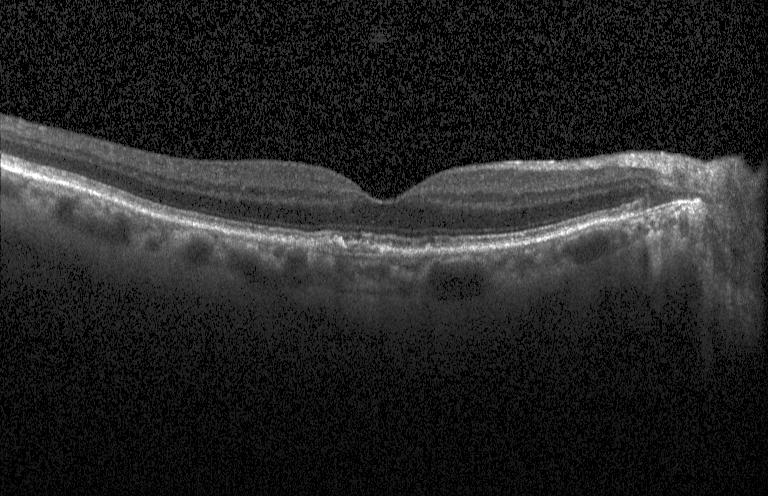

Retinal OCT cross-section showing multiple drusen.